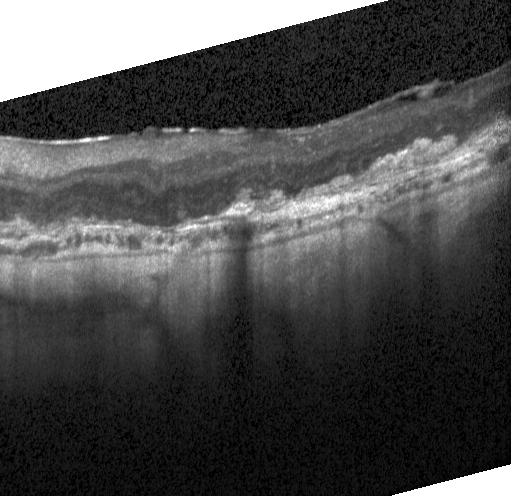
Retinal OCT cross-section; Heidelberg Spectralis OCT system — A choroidal neovascular membrane.